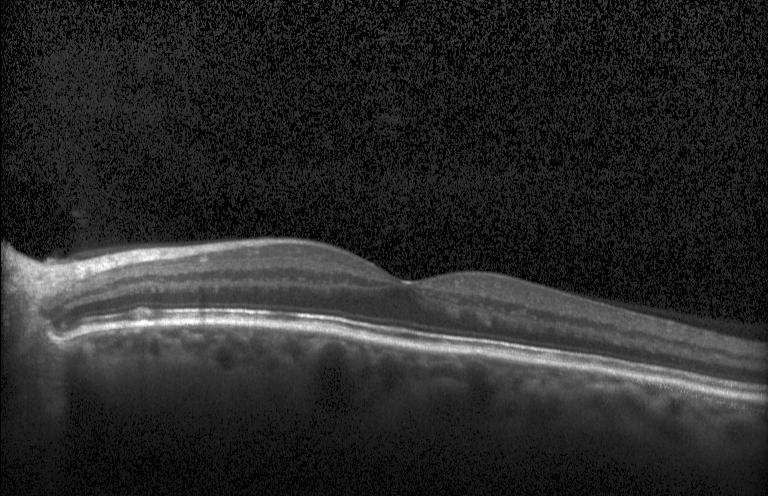
Optical coherence tomography scan. The scan shows no evidence of CNV, DME, or drusen.